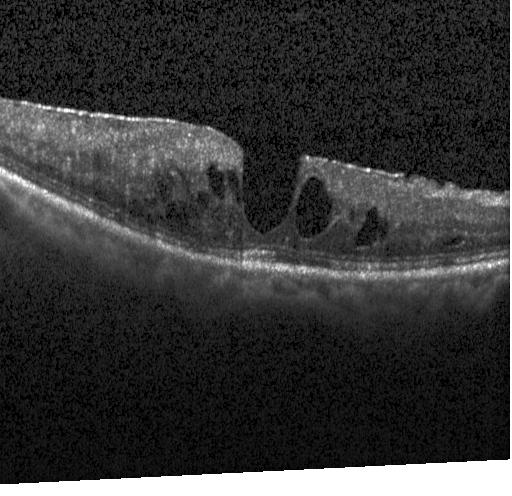
SD-OCT, fovea-centered, Heidelberg Spectralis OCT system, OCT line scan. Finding: diabetic macular edema (DME).